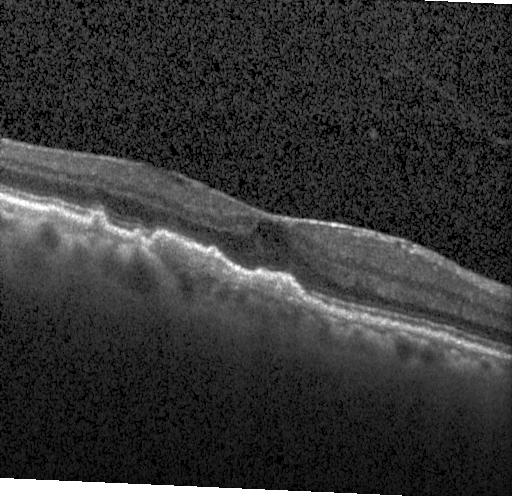 Retinal OCT B-scan — Assessment: a choroidal neovascular membrane.